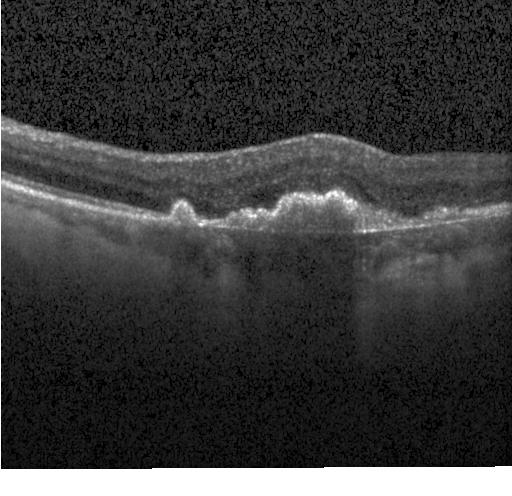
Optical coherence tomography scan. Assessment: a choroidal neovascular membrane.